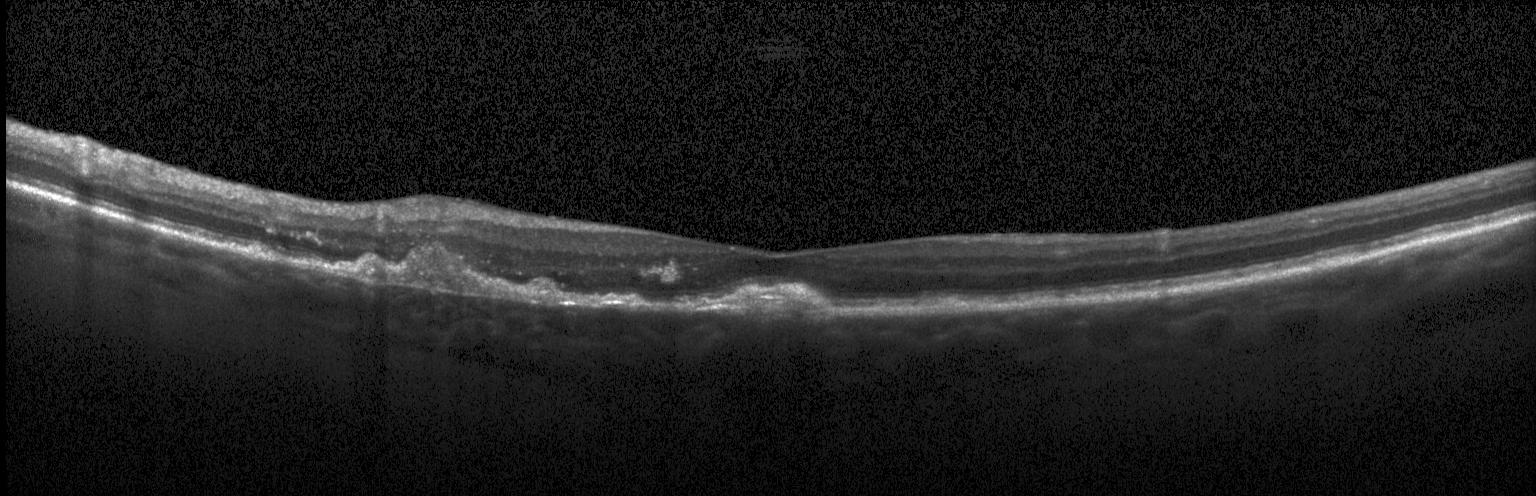 OCT scan showing a choroidal neovascular membrane.